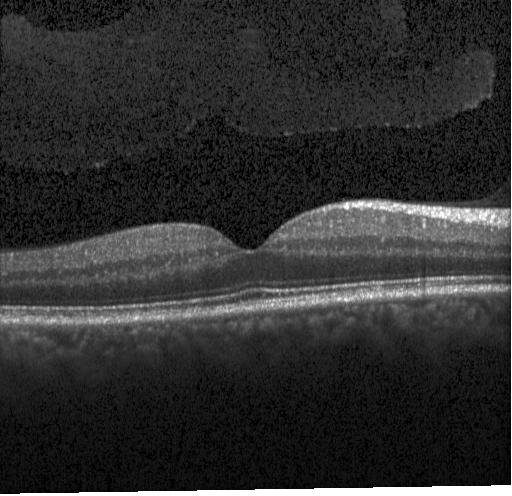 Retinal OCT cross-section, acquired on a Heidelberg Spectralis, through the macula, spectral-domain optical coherence tomography — No CNV, no DME, and no drusen.